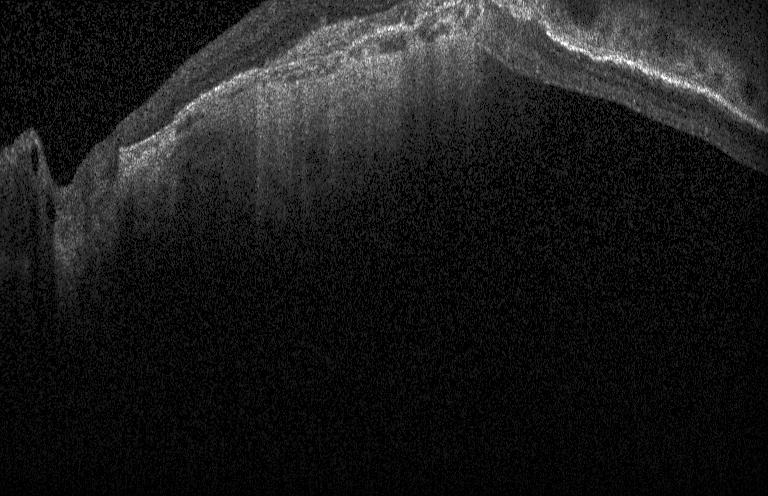
Spectral-domain OCT; retinal OCT B-scan; instrument: Heidelberg Spectralis; horizontal scan through the fovea.
Assessment: choroidal neovascularization (CNV).